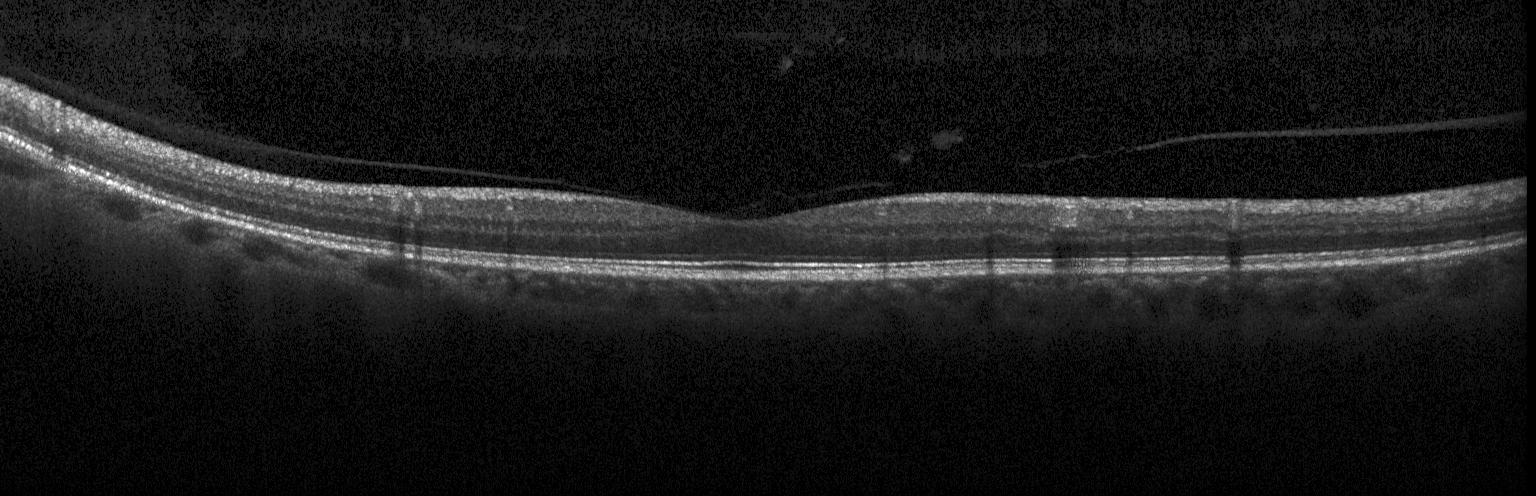 Retinal OCT B-scan — No evidence of choroidal neovascularization, diabetic macular edema, or drusen.